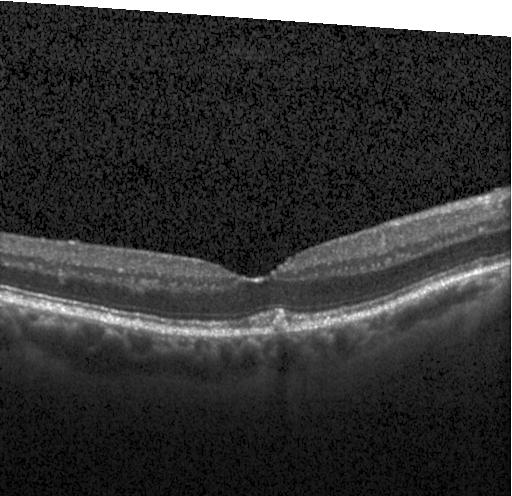
Optical coherence tomography scan. Finding: multiple drusen.